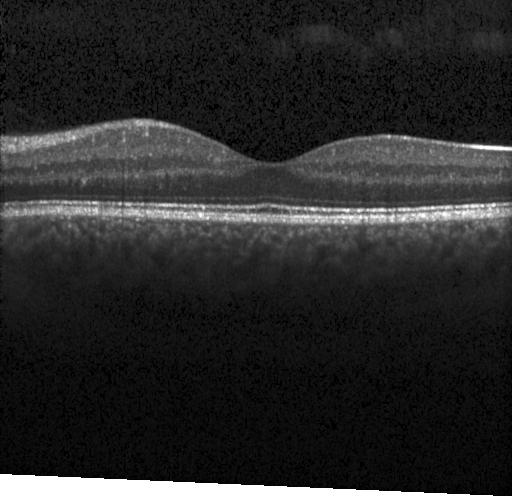
Impression: no evidence of choroidal neovascularization, diabetic macular edema, or drusen.